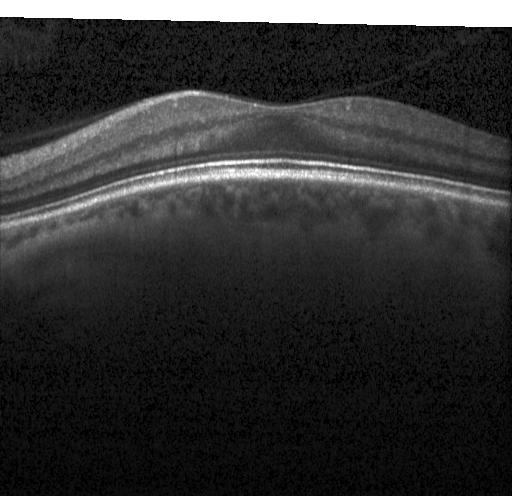

Finding: no evidence of choroidal neovascularization, diabetic macular edema, or drusen.